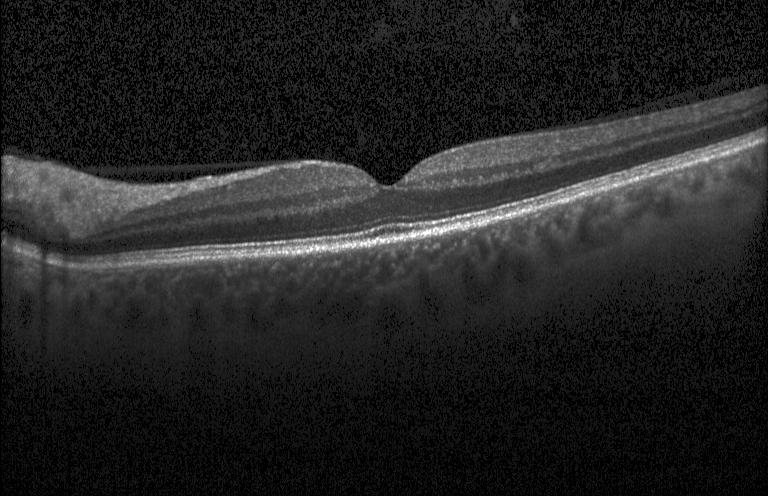 Optical coherence tomography scan
Diagnosis: neither choroidal neovascularization, diabetic macular edema, nor drusen.